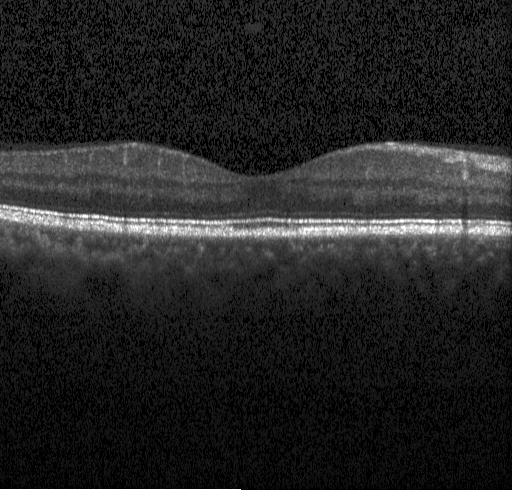 Heidelberg Spectralis OCT system. Optical coherence tomography B-scan. OCT finding: no choroidal neovascularization, no diabetic macular edema, and no drusen.